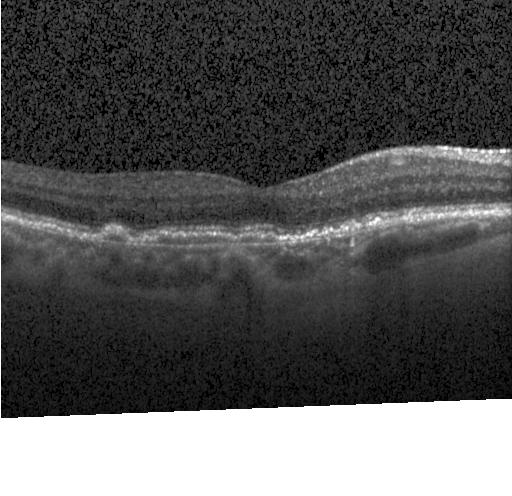

Diagnosis: choroidal neovascularization.